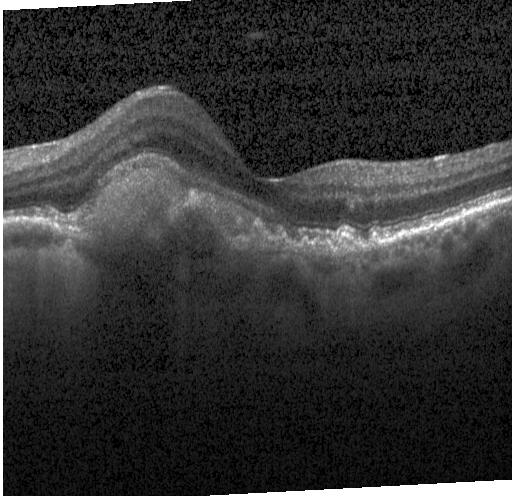 Fovea-centered · instrument: Heidelberg Spectralis · OCT B-scan · spectral-domain OCT
Diagnosis: a choroidal neovascular membrane.